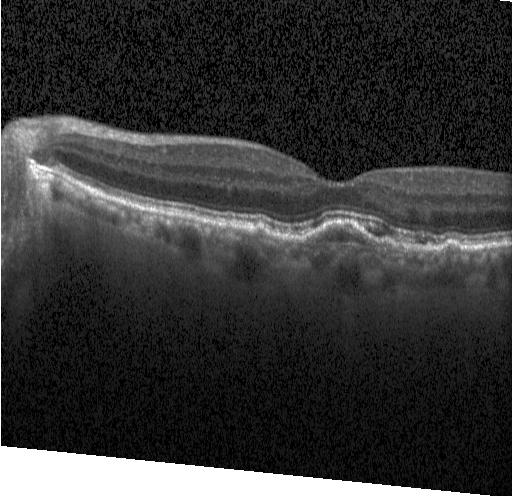 Finding: choroidal neovascularization.